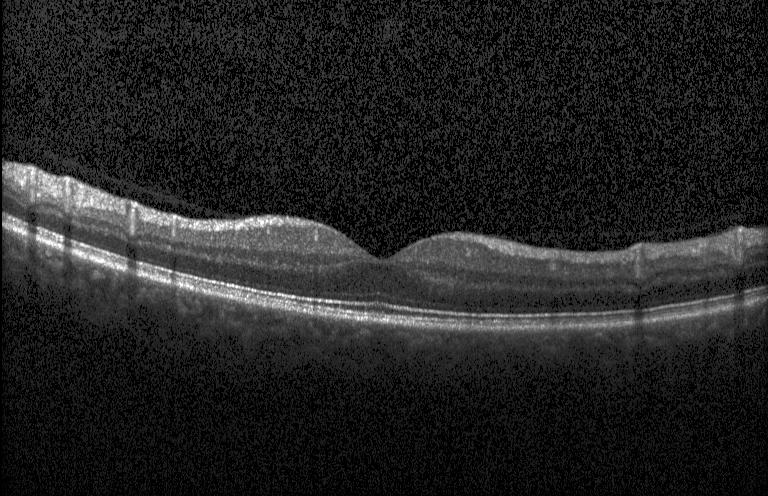

Retinal OCT cross-section
The scan shows no evidence of choroidal neovascularization, diabetic macular edema, or drusen.